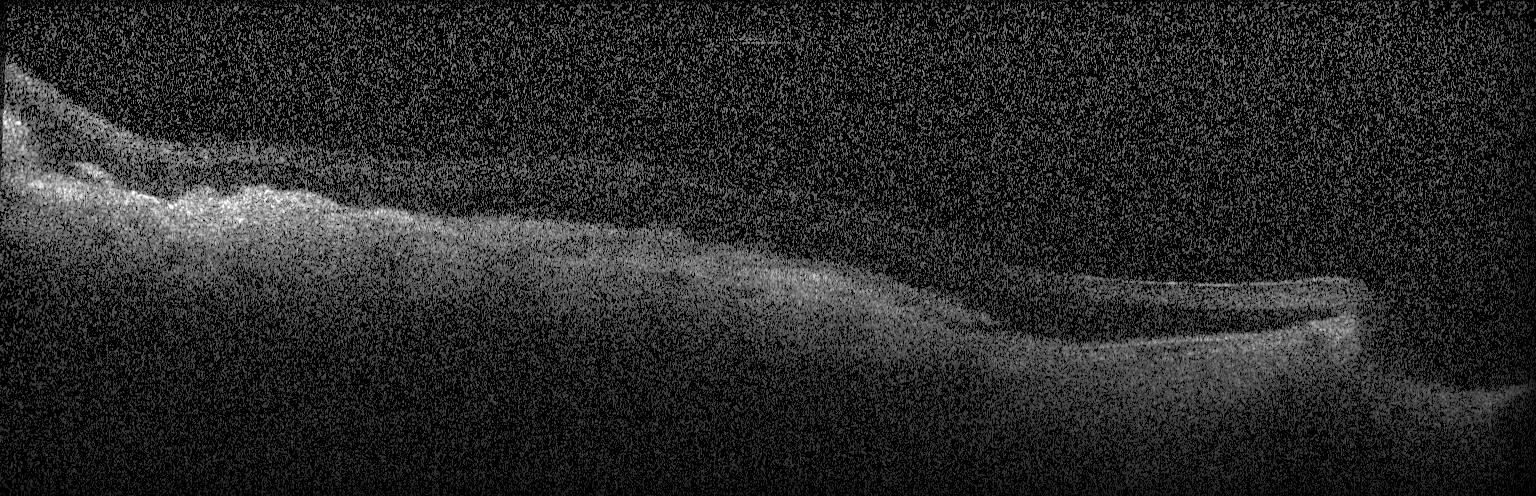 Optical coherence tomography scan · Heidelberg Spectralis. Finding: choroidal neovascularization.